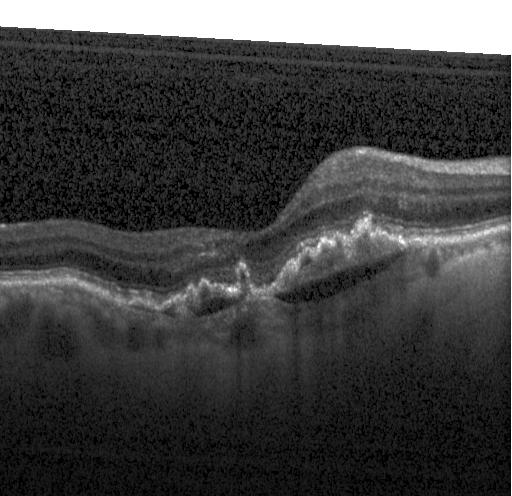

The scan shows a choroidal neovascular membrane.